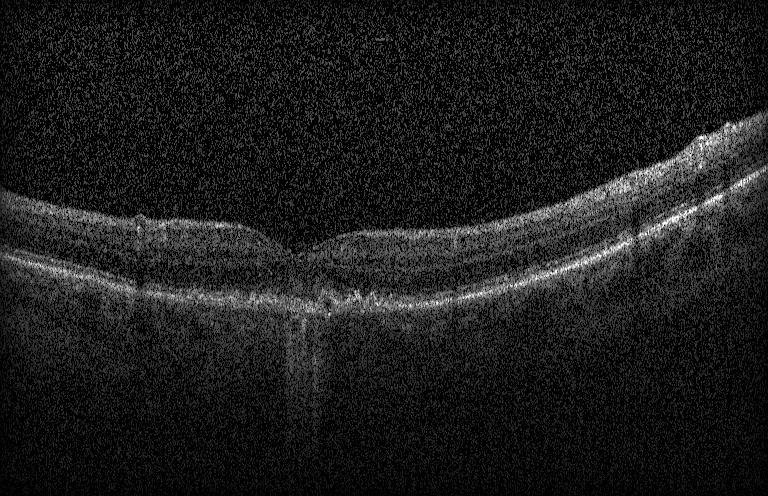
Spectral-domain OCT; Heidelberg Spectralis; fovea-centered; optical coherence tomography B-scan. Diagnosis: a choroidal neovascular membrane.